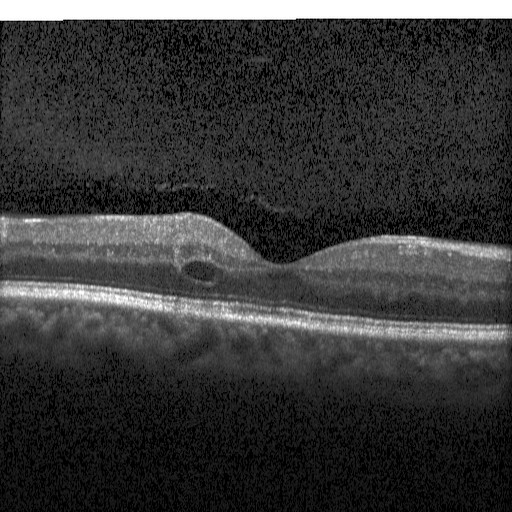
Retinal OCT cross-section.
Dx: diabetic macular edema (DME).